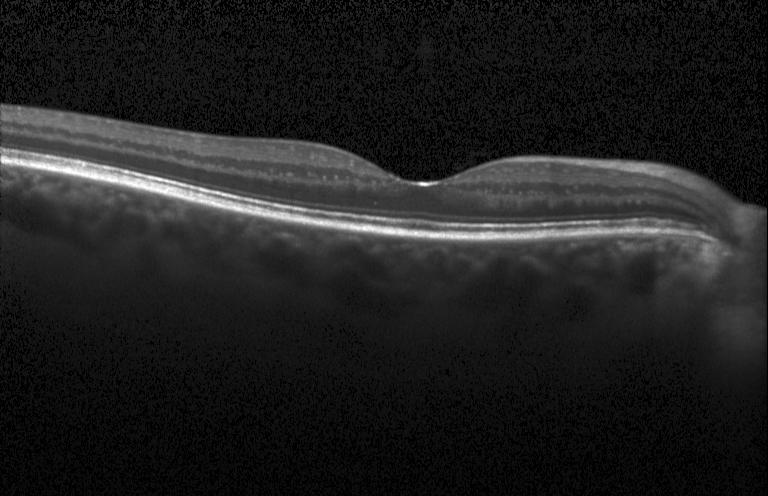

Retinal OCT cross-section.
Finding: no choroidal neovascularization, diabetic macular edema, or drusen.